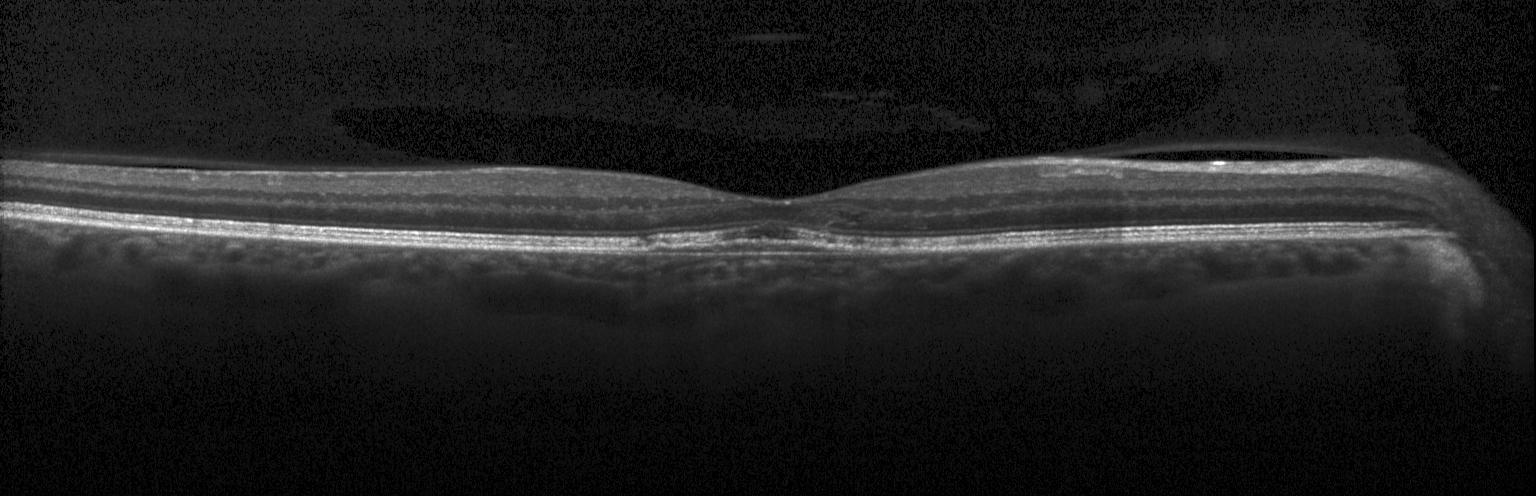

A choroidal neovascular membrane.